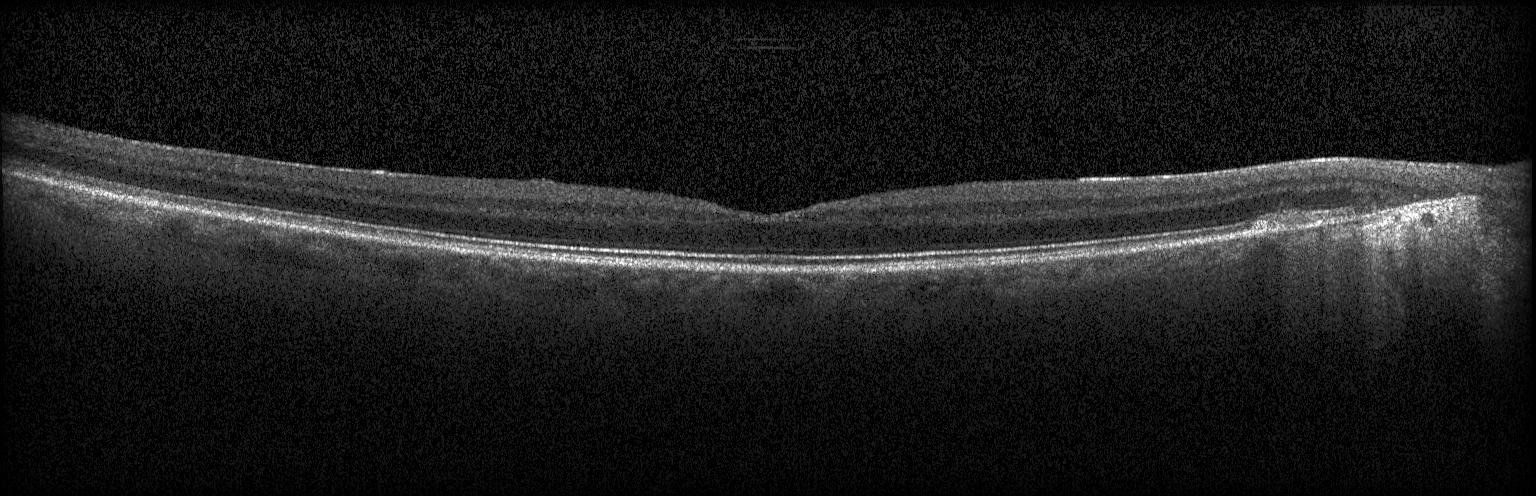
Retinal OCT B-scan, spectral-domain optical coherence tomography, instrument: Heidelberg Spectralis, macular scan — Macular OCT: no choroidal neovascularization, no diabetic macular edema, and no drusen.